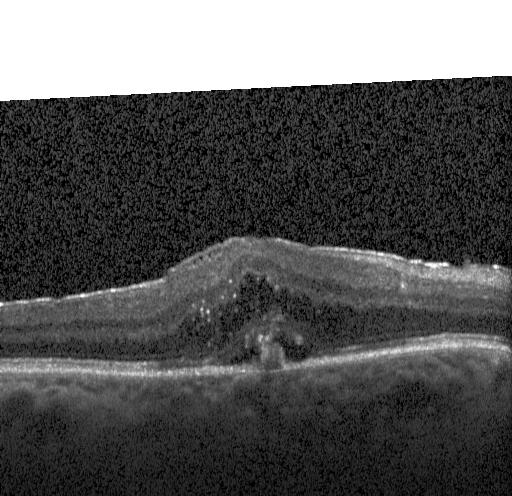

Assessment: choroidal neovascularization (CNV).